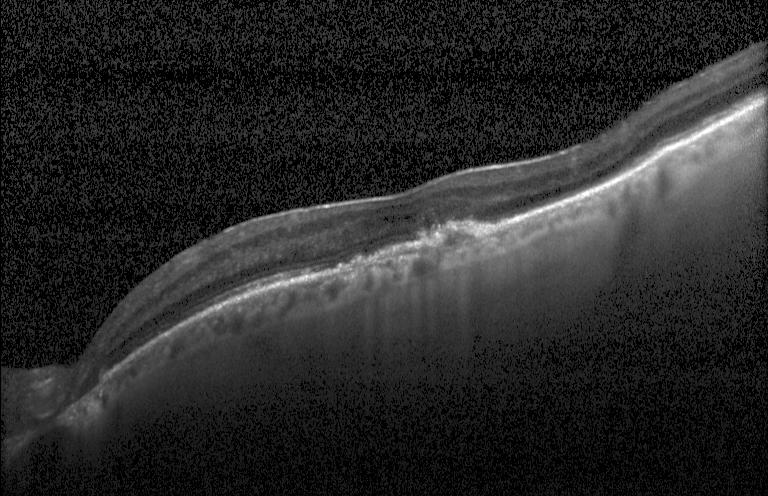
Retinal OCT cross-section — The scan shows a choroidal neovascular membrane.